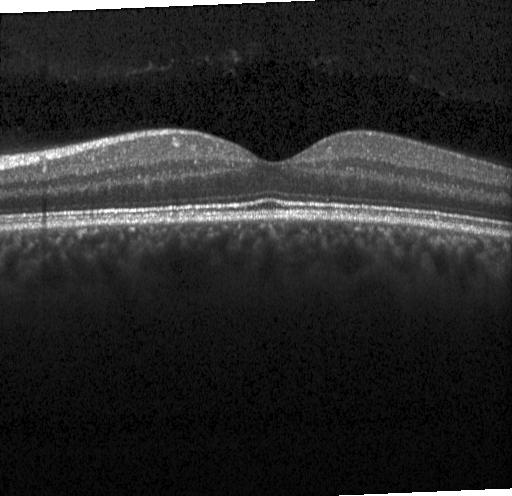 Spectral-domain OCT; acquired on a Heidelberg Spectralis; optical coherence tomography B-scan; fovea-centered
Diagnosis: no choroidal neovascularization, diabetic macular edema, or drusen.